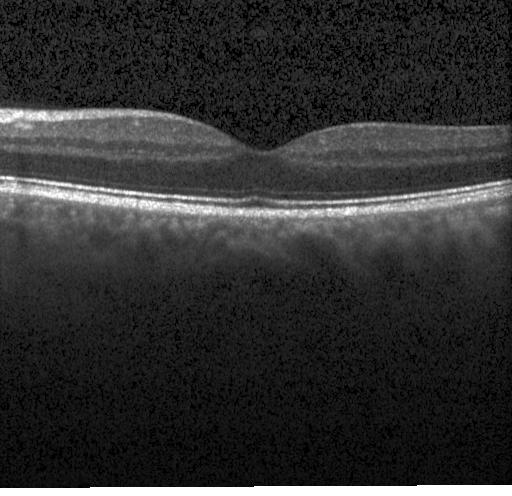 Impression: no evidence of choroidal neovascularization, diabetic macular edema, or drusen.